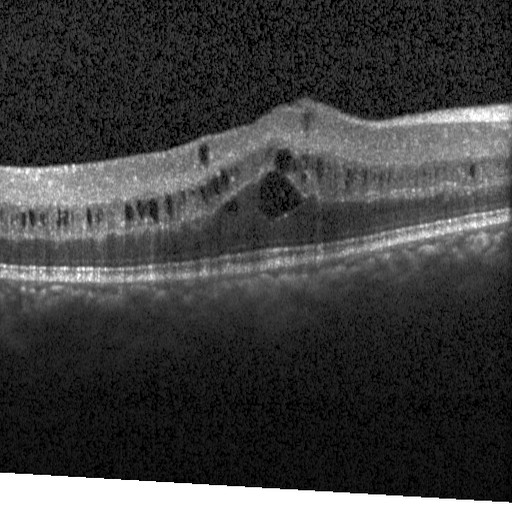

Fovea-centered · optical coherence tomography scan · instrument: Heidelberg Spectralis. The scan shows DME.